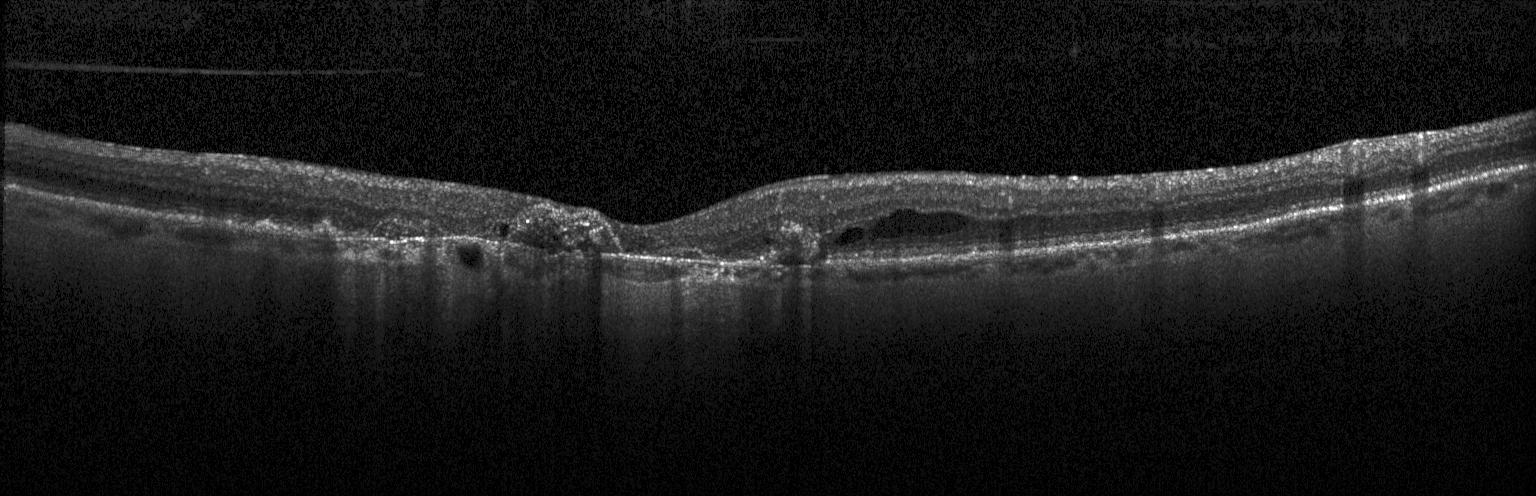

Spectral-domain optical coherence tomography; Heidelberg Spectralis OCT system; optical coherence tomography B-scan; through the macula — Impression: a choroidal neovascular membrane.